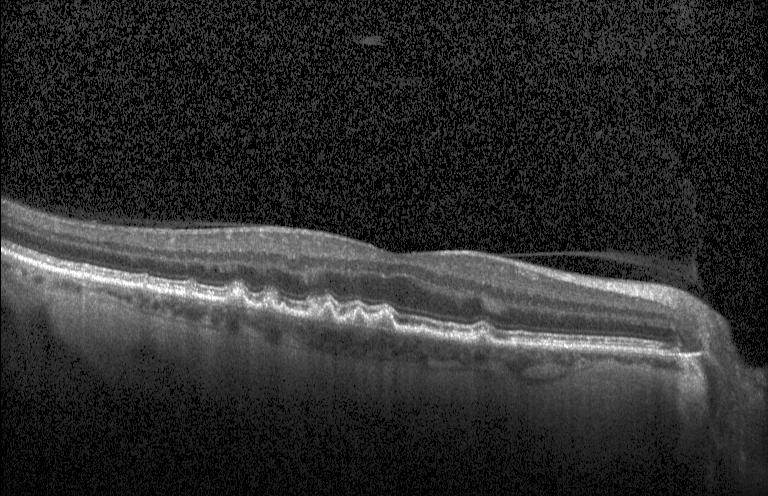
OCT B-scan. Heidelberg Spectralis.
Assessment: drusen.